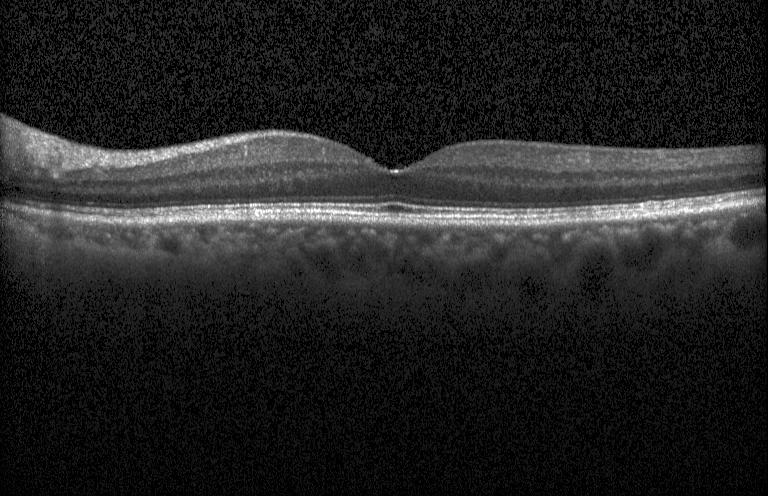
Retinal OCT cross-section · Heidelberg Spectralis · macular scan · SD-OCT.
Macular OCT: no evidence of CNV, DME, or drusen.